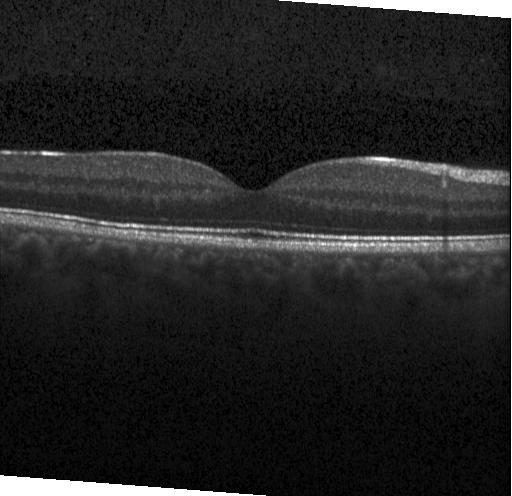 Diagnosis: no choroidal neovascularization, diabetic macular edema, or drusen.